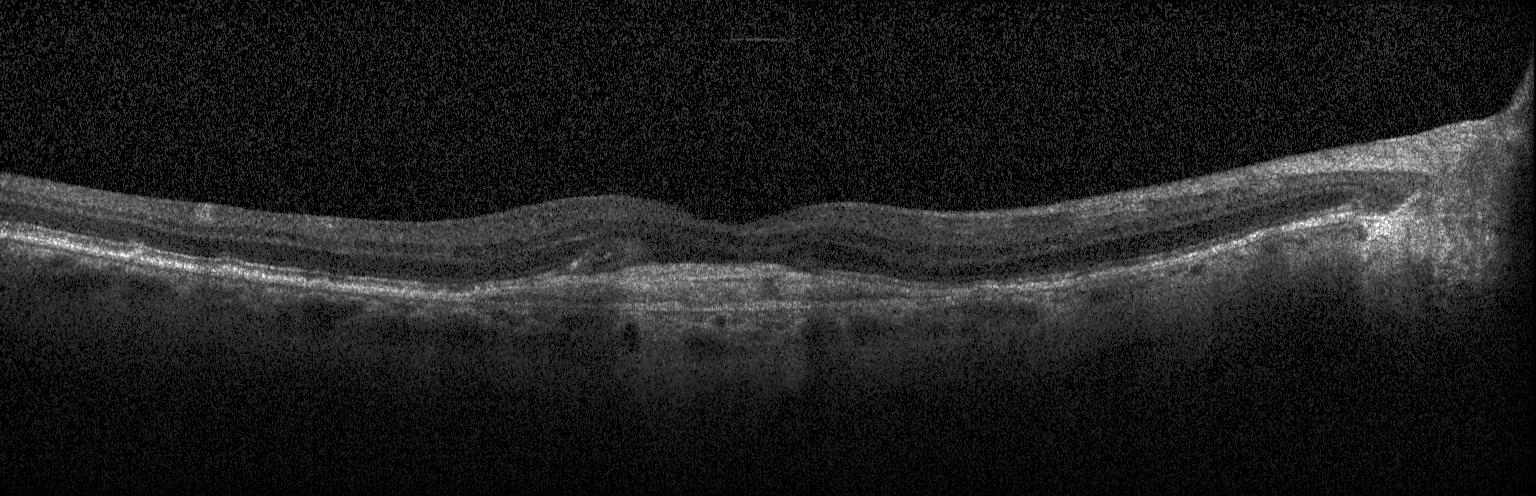
Finding: choroidal neovascularization.